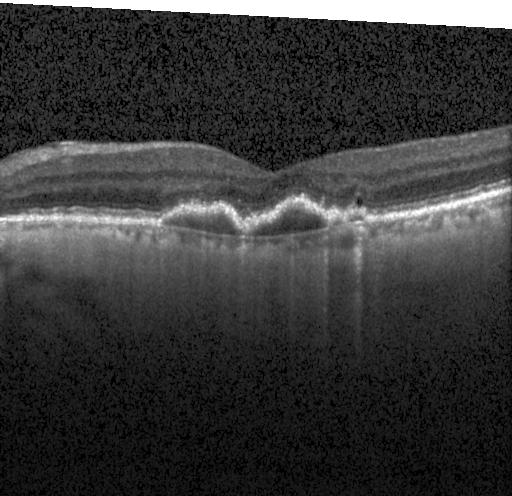 Retinal OCT B-scan · SD-OCT.
This B-scan demonstrates choroidal neovascularization.